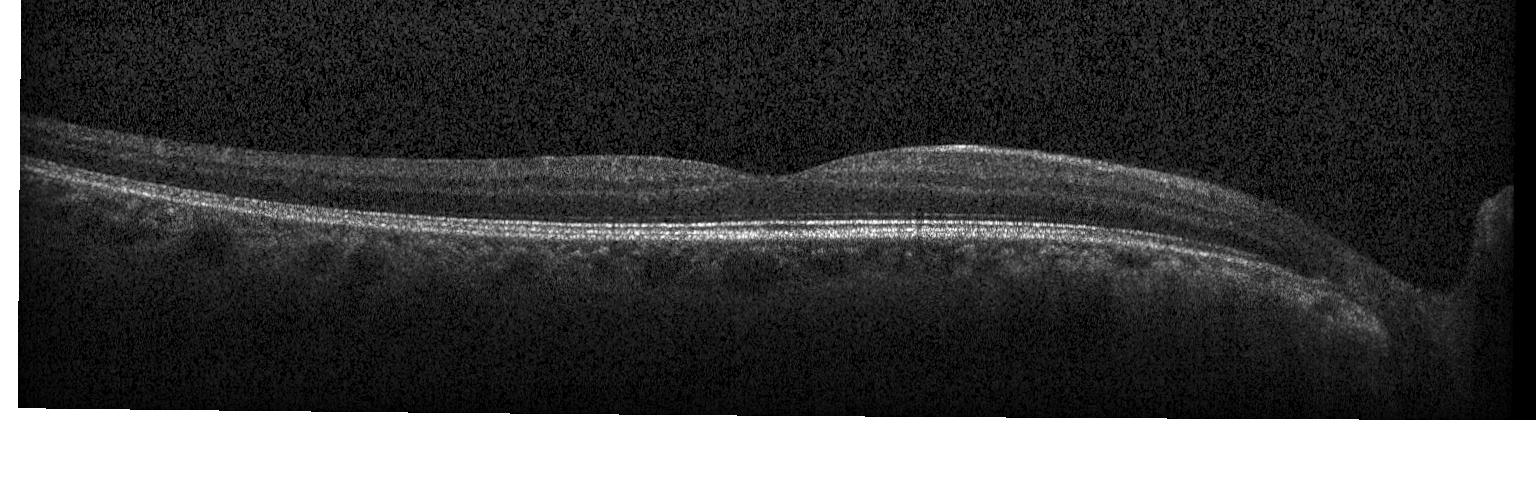
Diagnosis: no evidence of choroidal neovascularization, diabetic macular edema, or drusen.